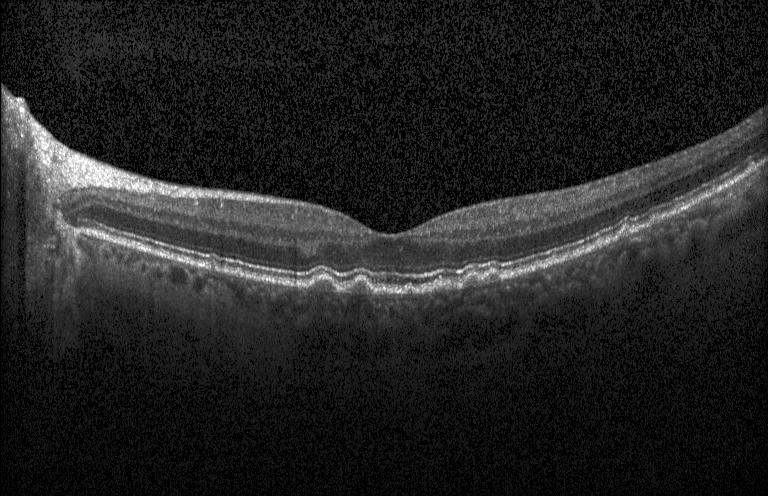
Through the macula, Heidelberg Spectralis OCT system, optical coherence tomography B-scan
Impression: drusen.